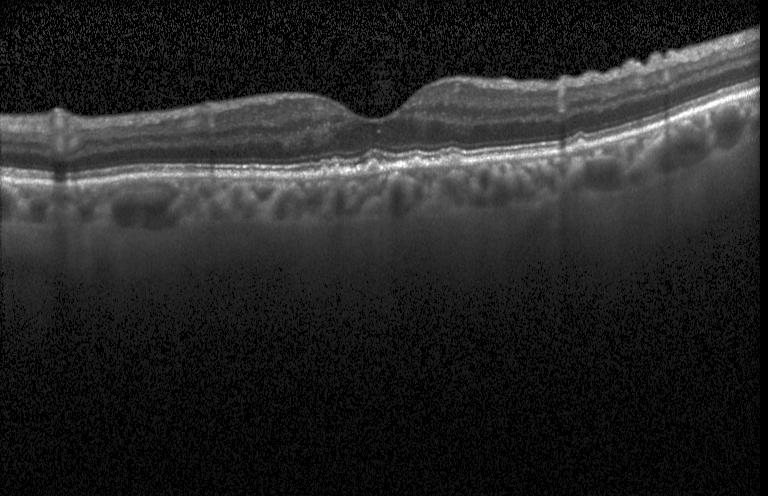
OCT scan showing multiple drusen.